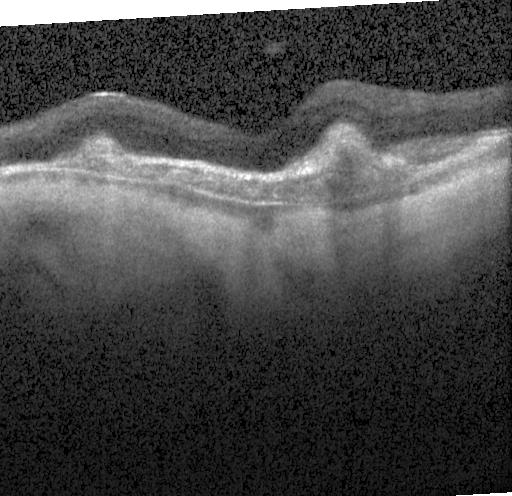

OCT scan showing choroidal neovascularization.